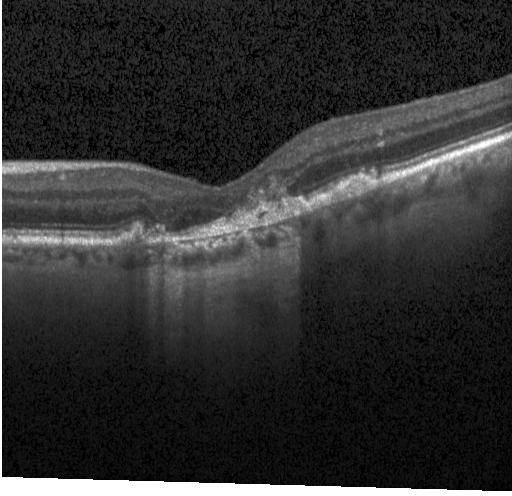

Through the macula · optical coherence tomography scan · spectral-domain optical coherence tomography — CNV.